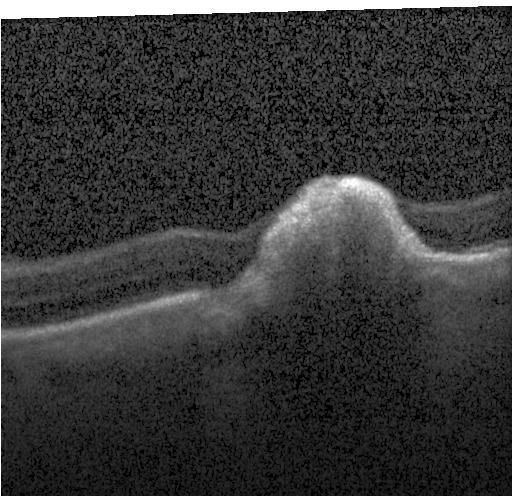
OCT B-scan.
This B-scan demonstrates choroidal neovascularization.